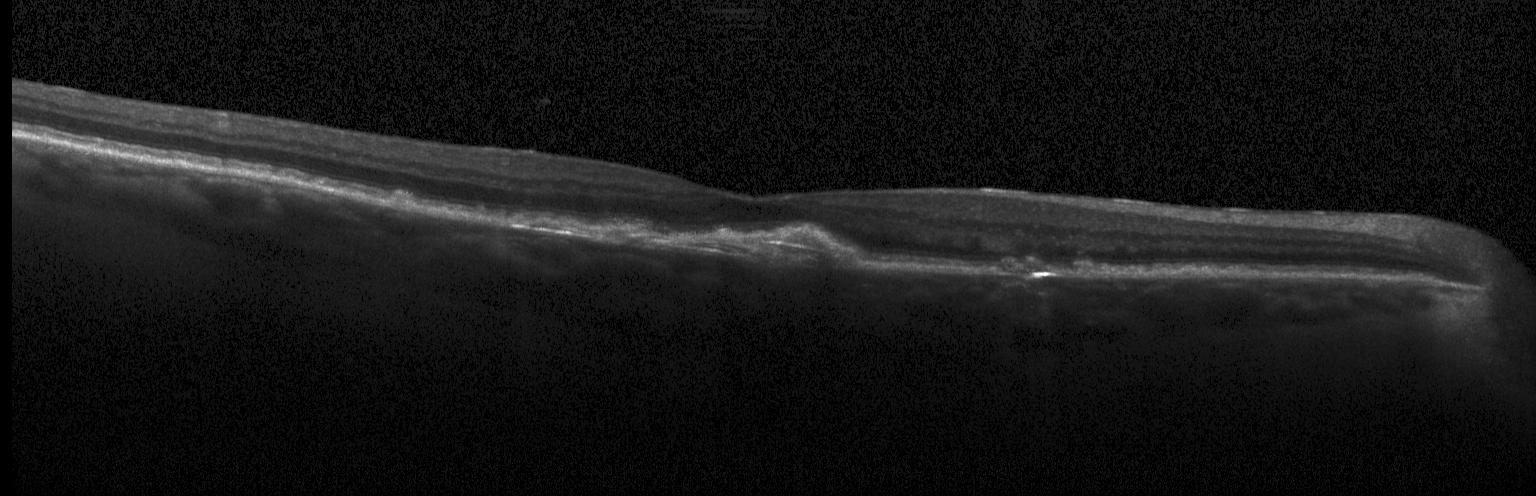
Macular OCT demonstrating CNV.